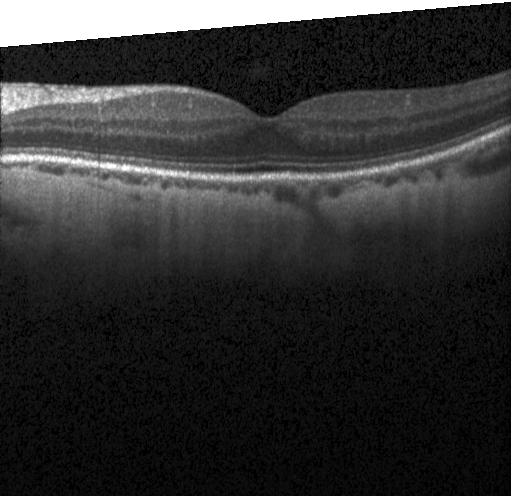

Assessment: no choroidal neovascularization, no diabetic macular edema, and no drusen.